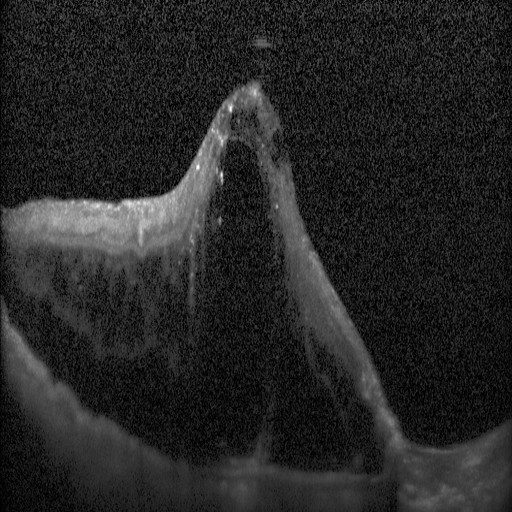 SD-OCT, optical coherence tomography B-scan
Diagnosis: diabetic macular edema (DME).